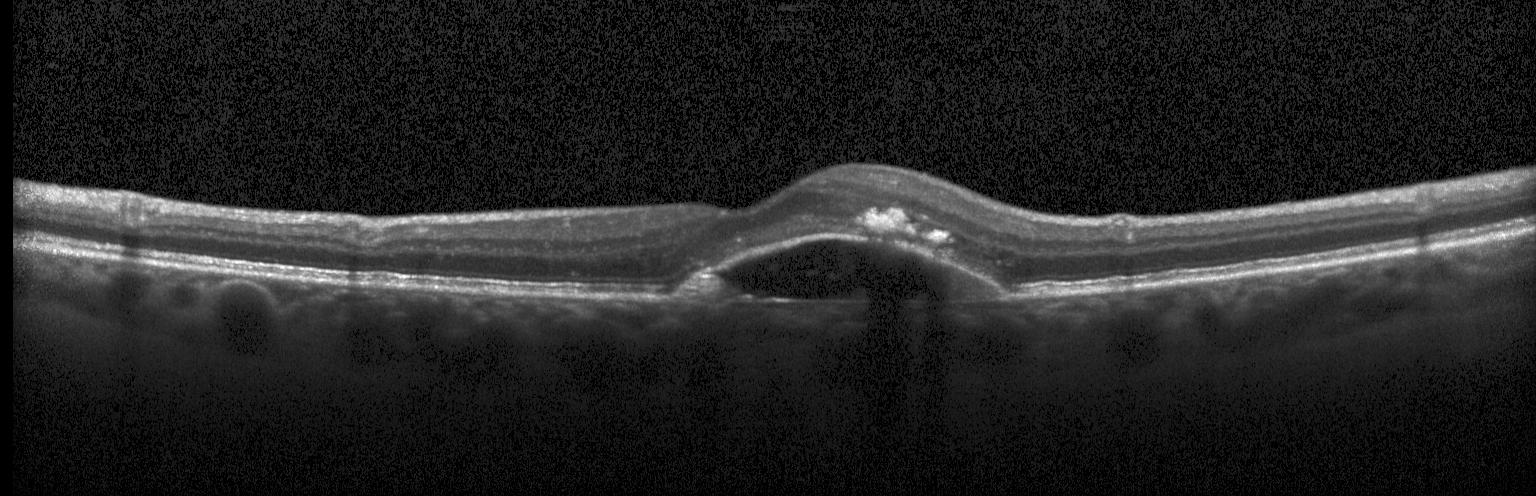
OCT finding: a choroidal neovascular membrane.